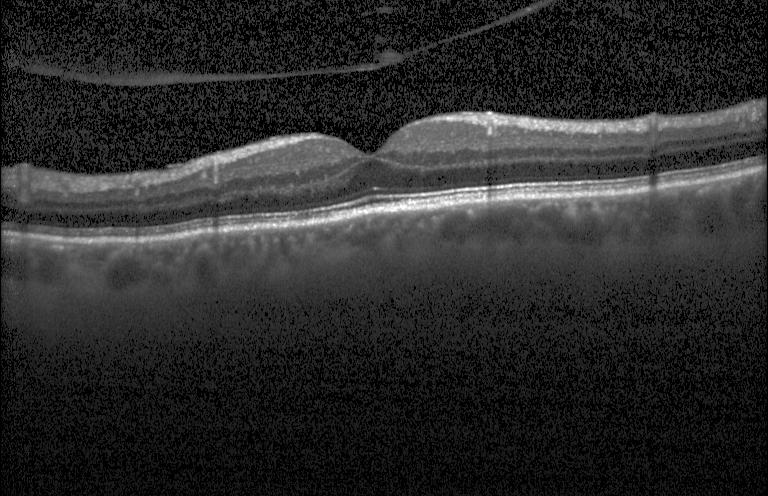
Acquired on a Heidelberg Spectralis. Centered on the fovea. OCT line scan. Spectral-domain optical coherence tomography. Diagnosis: neither choroidal neovascularization, diabetic macular edema, nor drusen.